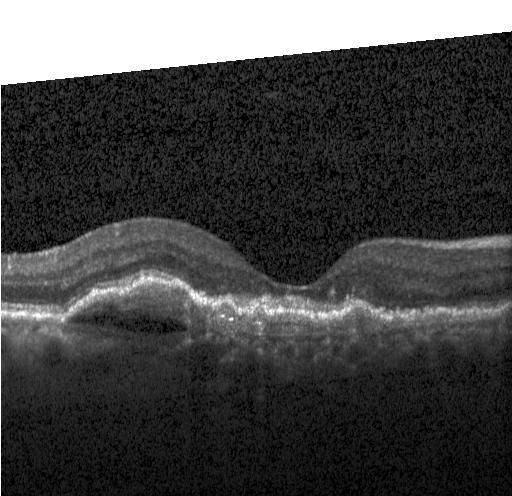
Spectral-domain optical coherence tomography · macular scan · optical coherence tomography B-scan · Heidelberg Spectralis OCT system. This B-scan demonstrates choroidal neovascularization.